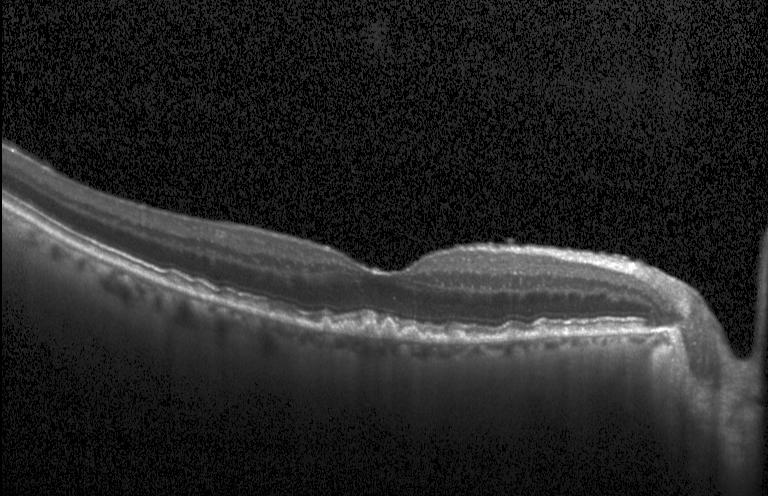 SD-OCT, Heidelberg Spectralis, retinal OCT B-scan, horizontal scan through the fovea — Finding: sub-RPE drusenoid deposits.